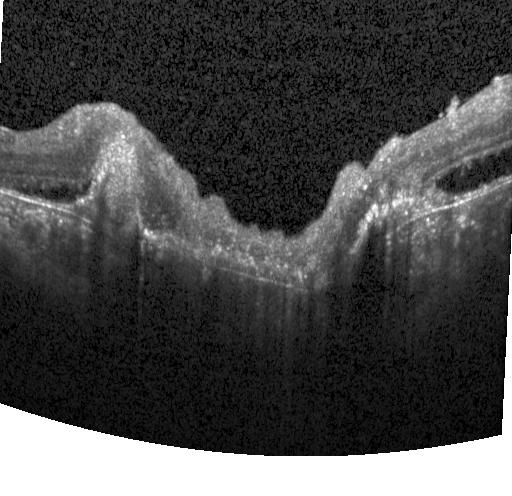

Diagnosis: a choroidal neovascular membrane.